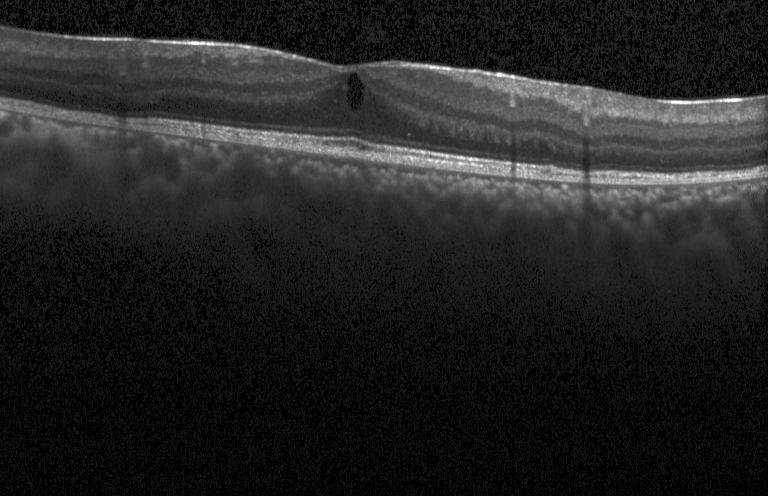

OCT line scan. Impression: DME.